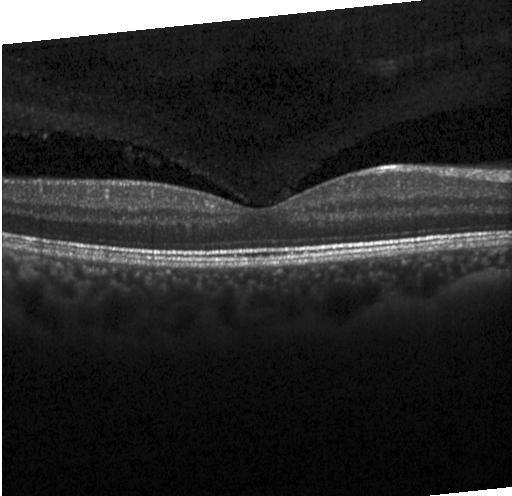
OCT B-scan. Finding: neither choroidal neovascularization, diabetic macular edema, nor drusen.